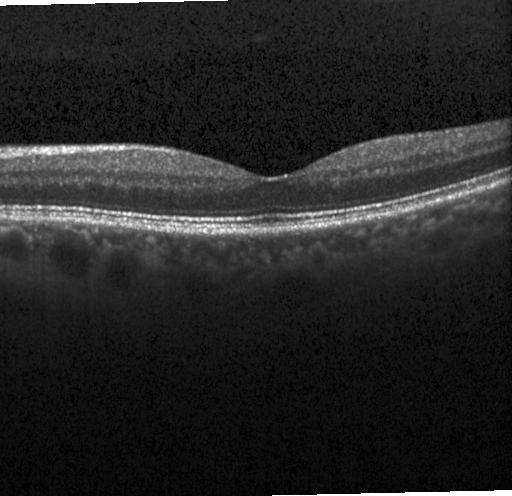 Instrument: Heidelberg Spectralis; OCT B-scan.
Impression: neither CNV, DME, nor drusen.